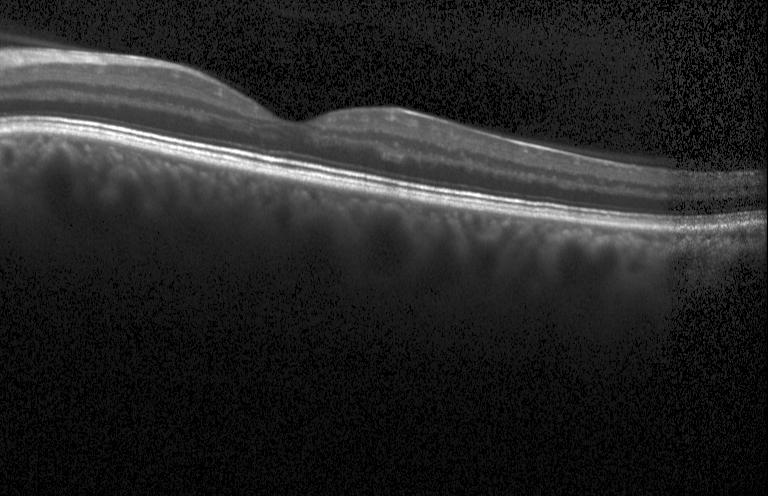

Finding: no choroidal neovascularization, diabetic macular edema, or drusen.